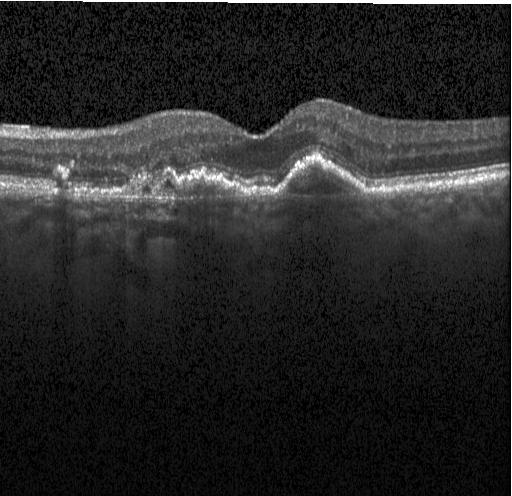 Instrument: Heidelberg Spectralis; OCT line scan — Macular OCT: a choroidal neovascular membrane.